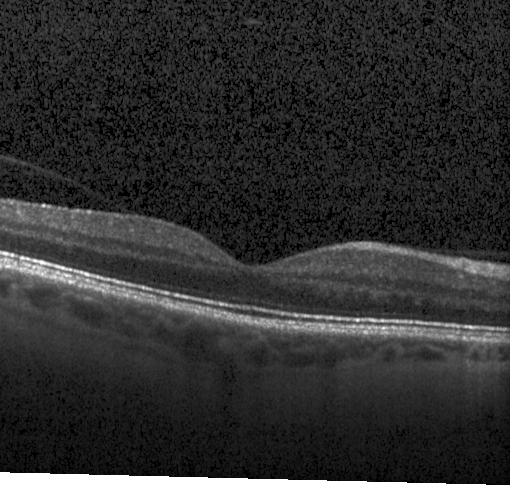 Macular OCT: neither CNV, DME, nor drusen.